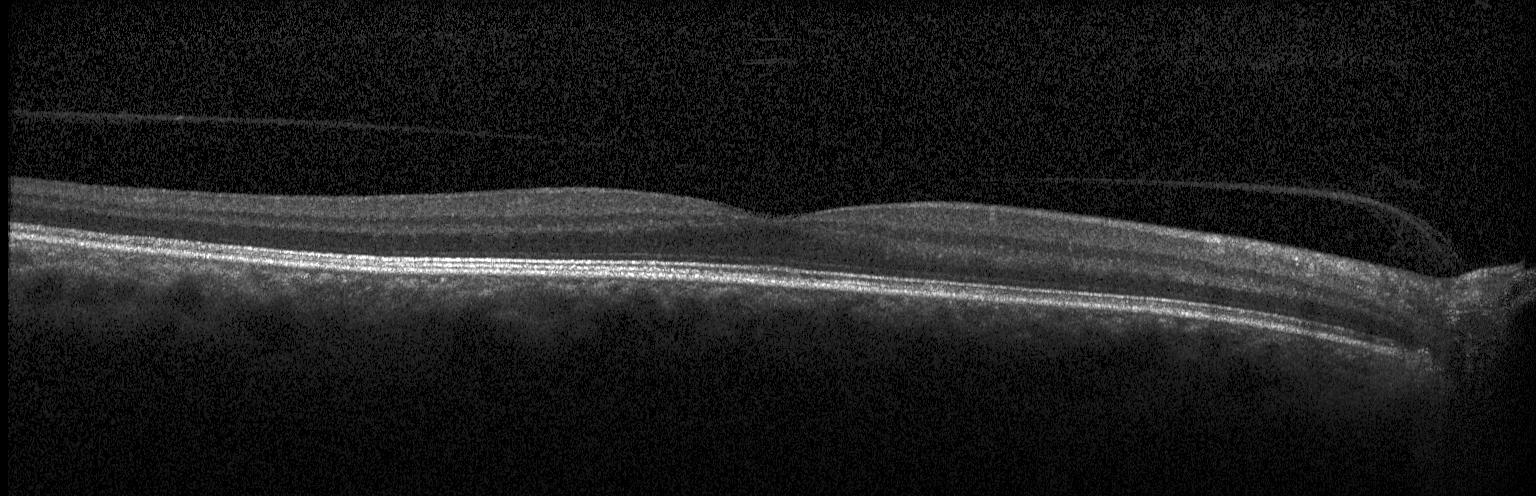
Macular OCT: neither choroidal neovascularization, diabetic macular edema, nor drusen.